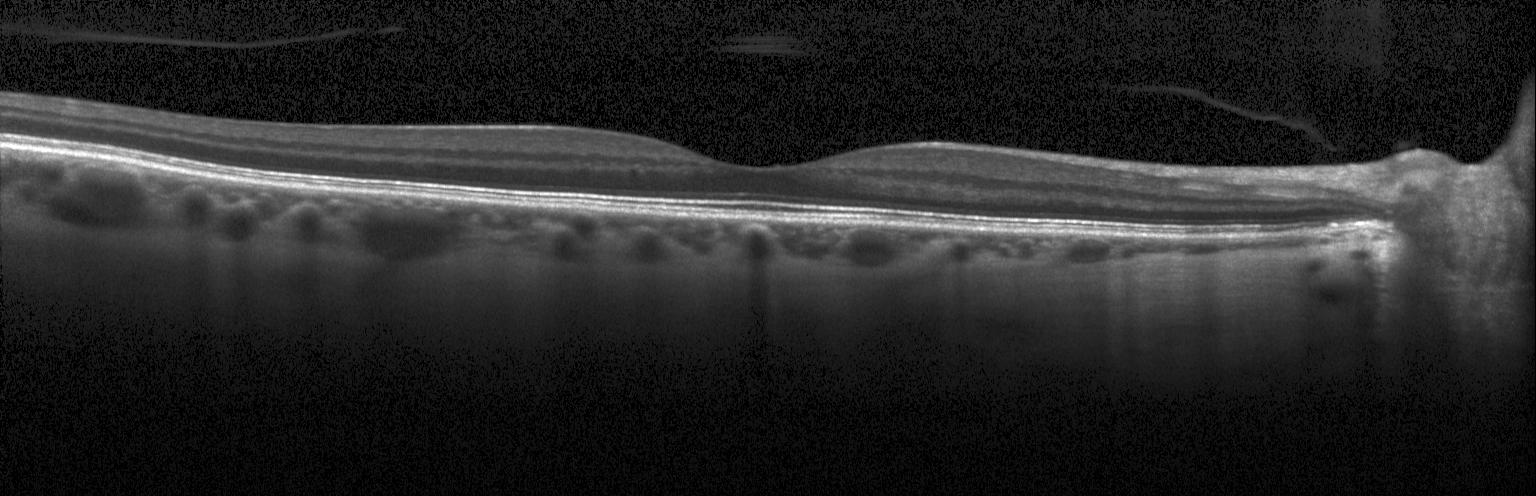

Impression: no evidence of CNV, DME, or drusen.